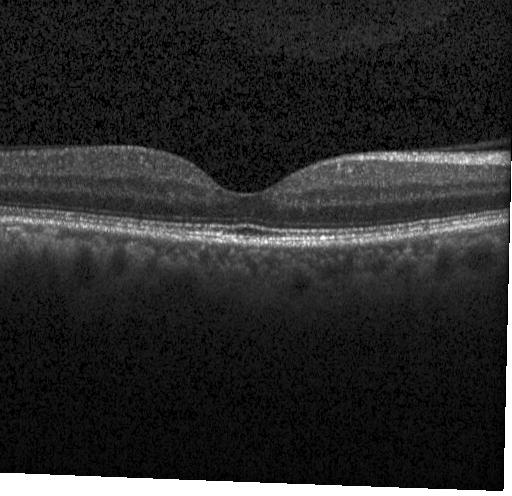 Finding: no choroidal neovascularization, diabetic macular edema, or drusen.